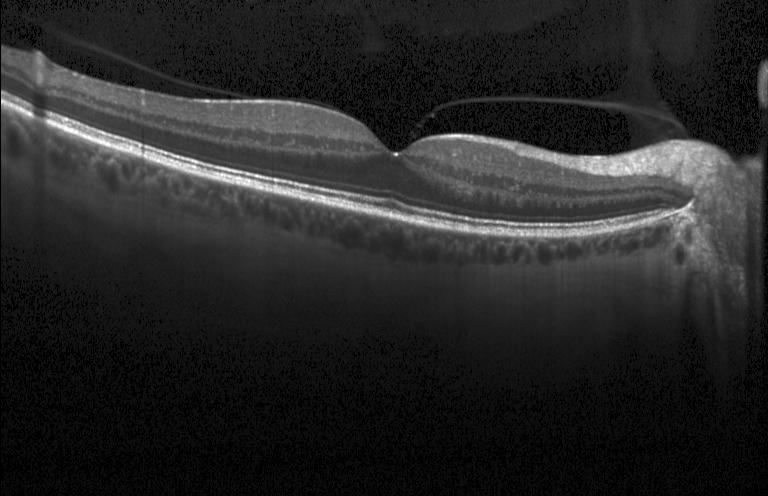

Impression: neither CNV, DME, nor drusen.